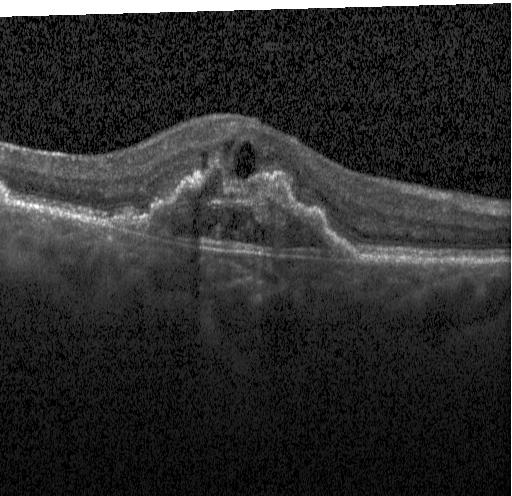

Retinal OCT cross-section showing a choroidal neovascular membrane.